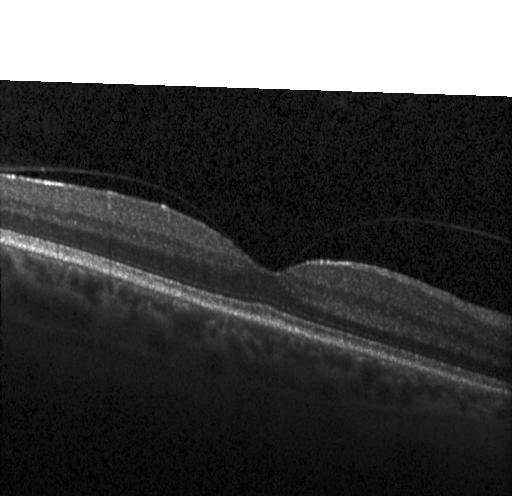

Spectral-domain OCT · OCT B-scan · through the macula · instrument: Heidelberg Spectralis — OCT finding: neither choroidal neovascularization, diabetic macular edema, nor drusen.